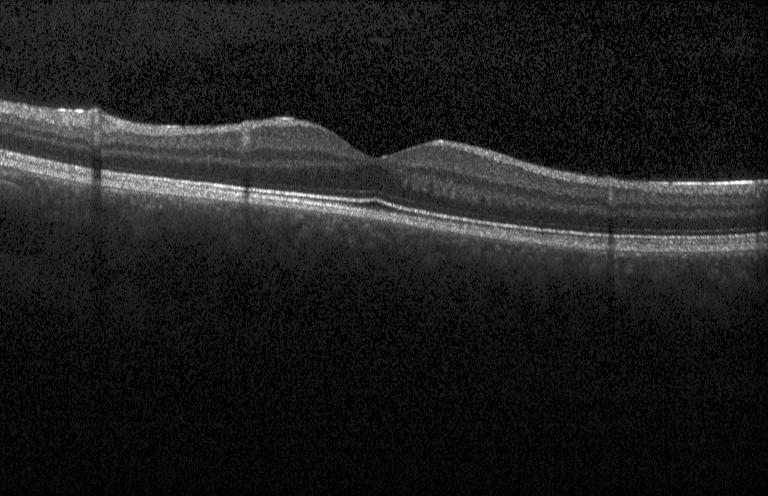

Retinal OCT B-scan. Horizontal scan through the fovea. Heidelberg Spectralis
Diagnosis: no CNV, no DME, and no drusen.